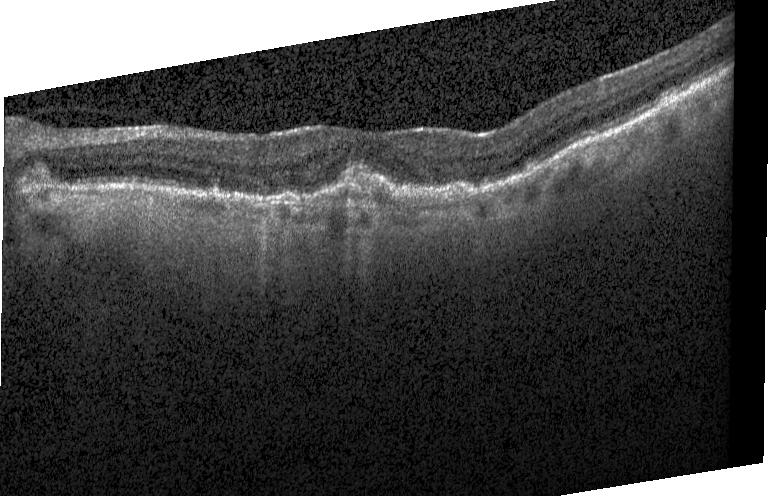
Centered on the fovea, OCT B-scan — OCT finding: a choroidal neovascular membrane.